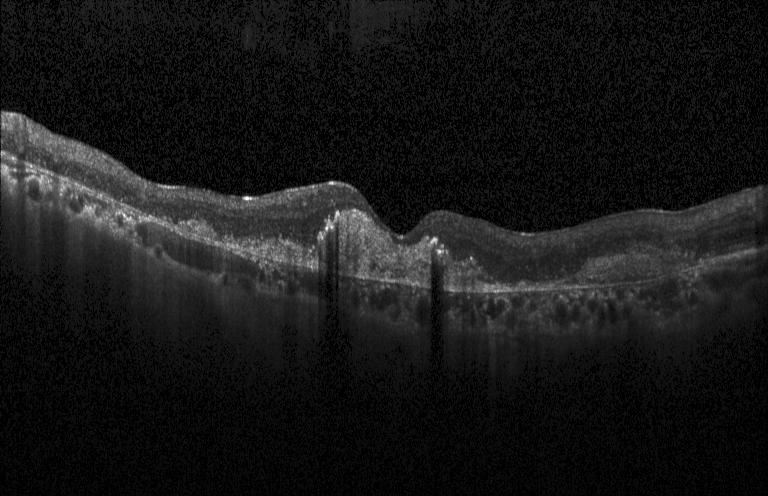 Heidelberg Spectralis; optical coherence tomography B-scan — Assessment: CNV.